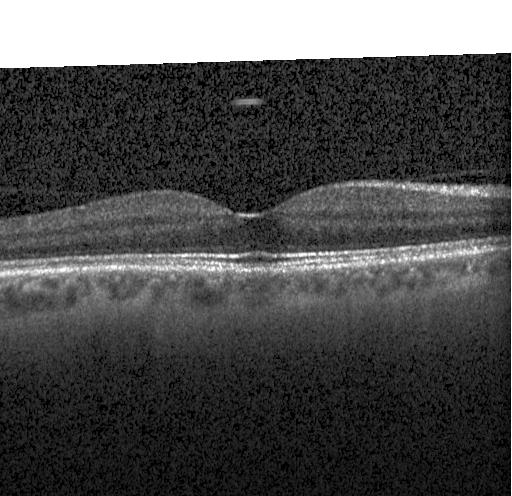
Heidelberg Spectralis. Through the macula. OCT B-scan. SD-OCT — Assessment: no CNV, no DME, and no drusen.